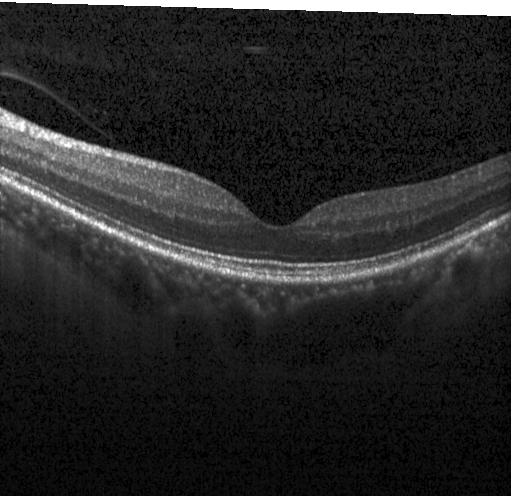
Spectral-domain OCT · macular scan · instrument: Heidelberg Spectralis · OCT B-scan.
Diagnosis: no choroidal neovascularization, diabetic macular edema, or drusen.